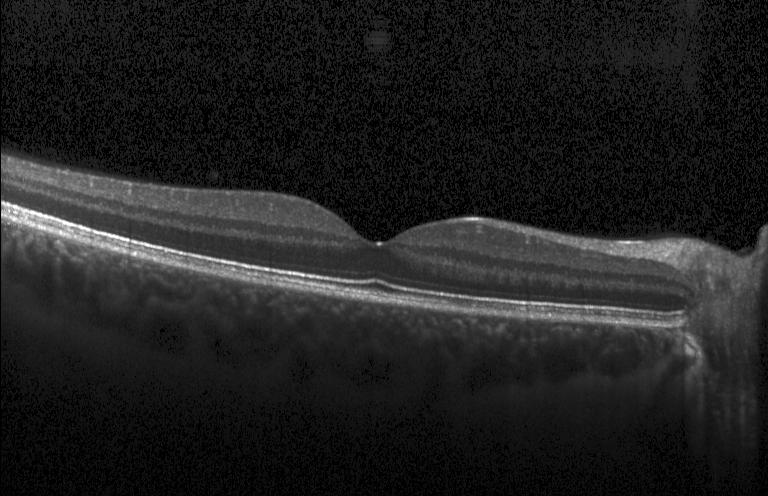
Heidelberg Spectralis OCT system · SD-OCT · optical coherence tomography B-scan · through the macula. Diagnosis: no evidence of choroidal neovascularization, diabetic macular edema, or drusen.